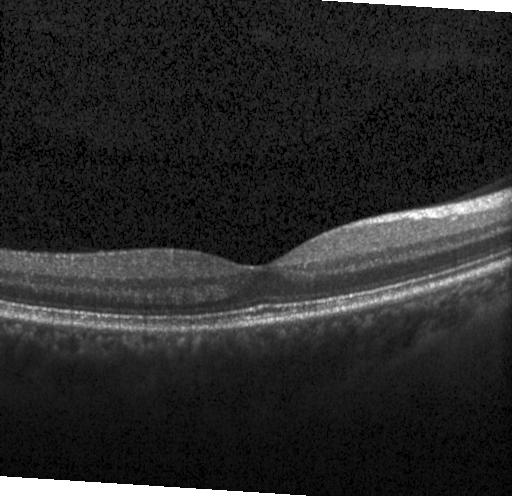 Finding: no evidence of choroidal neovascularization, diabetic macular edema, or drusen.